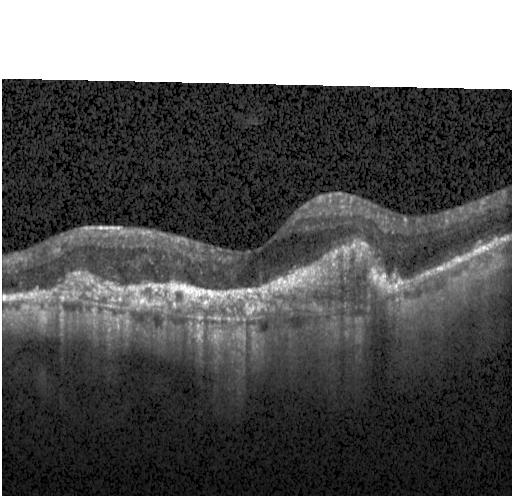
Through the macula. OCT line scan. Heidelberg Spectralis. The scan shows choroidal neovascularization (CNV).